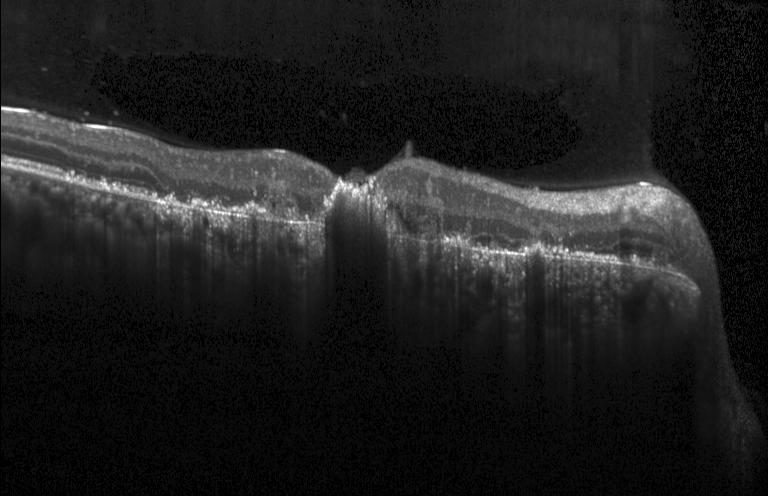 Finding: choroidal neovascularization (CNV).